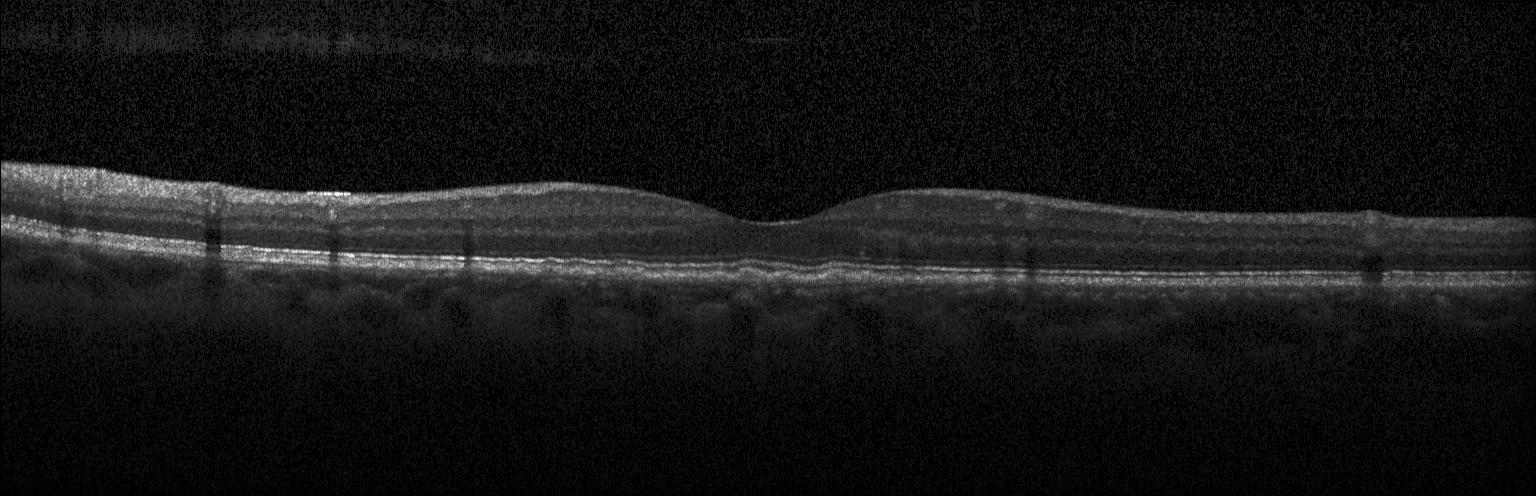

Impression: sub-RPE drusenoid deposits.